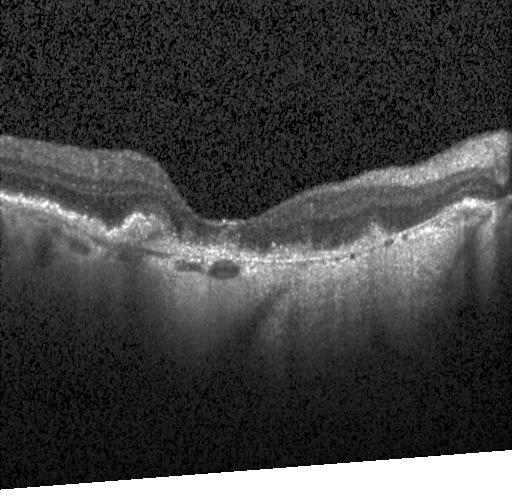

Dx: a choroidal neovascular membrane.